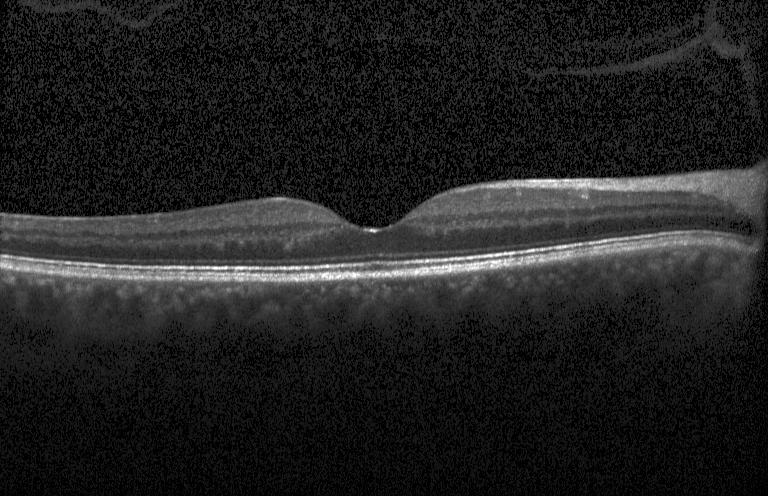 Acquired on a Heidelberg Spectralis; optical coherence tomography B-scan; horizontal scan through the fovea.
Impression: no choroidal neovascularization, no diabetic macular edema, and no drusen.